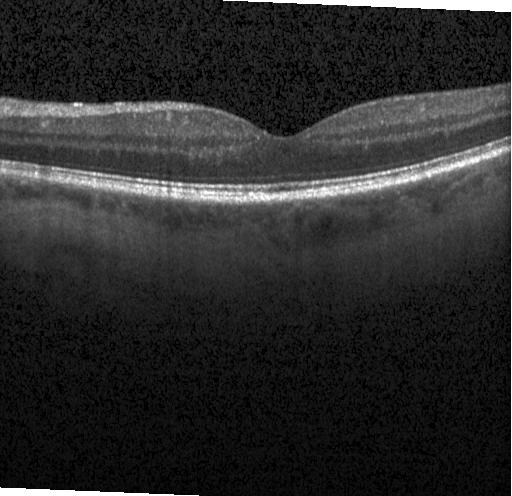
Macular OCT demonstrating no choroidal neovascularization, diabetic macular edema, or drusen.